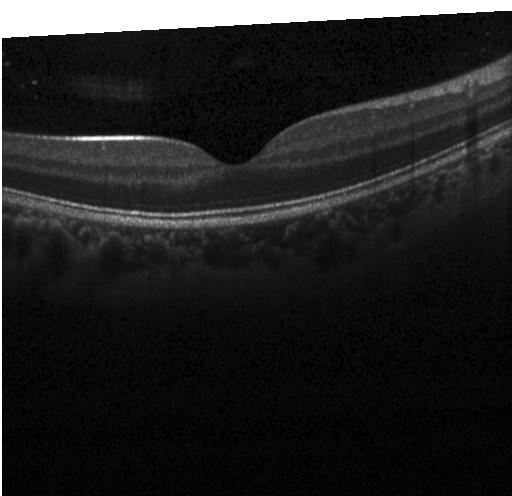
SD-OCT, optical coherence tomography scan, horizontal scan through the fovea.
Finding: no CNV, DME, or drusen.